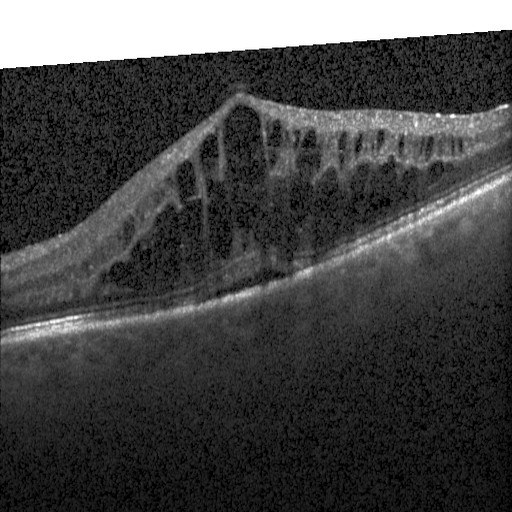 Optical coherence tomography scan — Assessment: diabetic macular edema (DME).